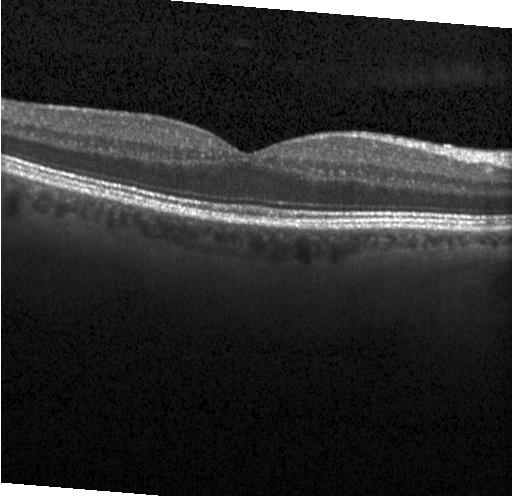 Optical coherence tomography B-scan. Heidelberg Spectralis OCT system. Spectral-domain optical coherence tomography. Macular scan
Assessment: no CNV, no DME, and no drusen.